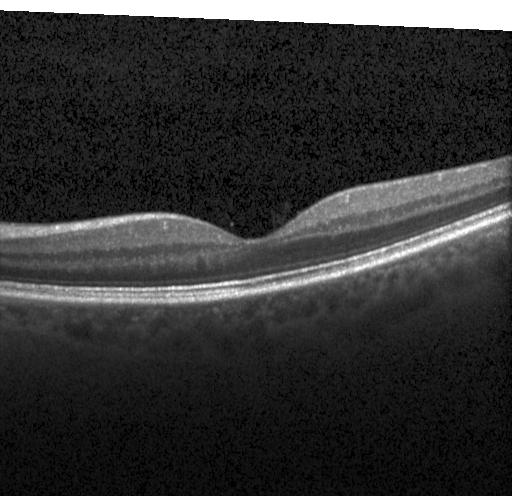 Spectral-domain OCT B-scan: neither choroidal neovascularization, diabetic macular edema, nor drusen.